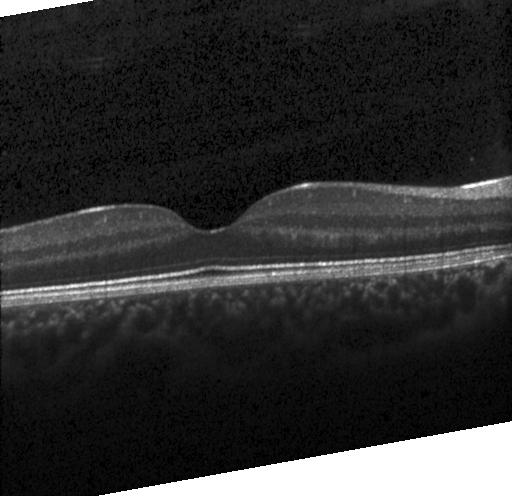

Horizontal scan through the fovea · Heidelberg Spectralis · OCT line scan.
Finding: no choroidal neovascularization, diabetic macular edema, or drusen.